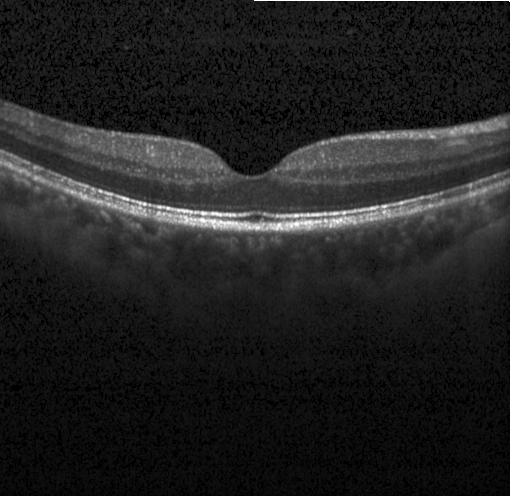 Finding: no CNV, no DME, and no drusen.